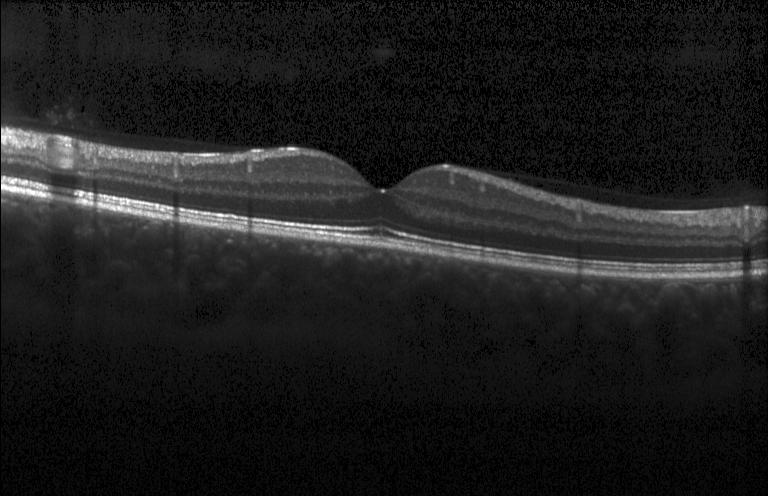 Retinal OCT cross-section · Heidelberg Spectralis OCT system. OCT finding: neither CNV, DME, nor drusen.